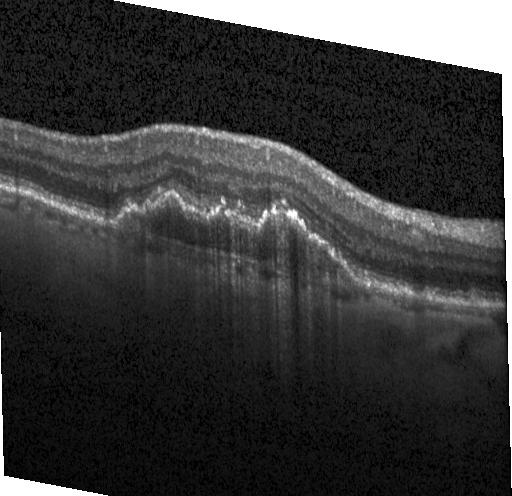
Horizontal scan through the fovea · acquired on a Heidelberg Spectralis · SD-OCT · OCT B-scan — Dx: CNV.